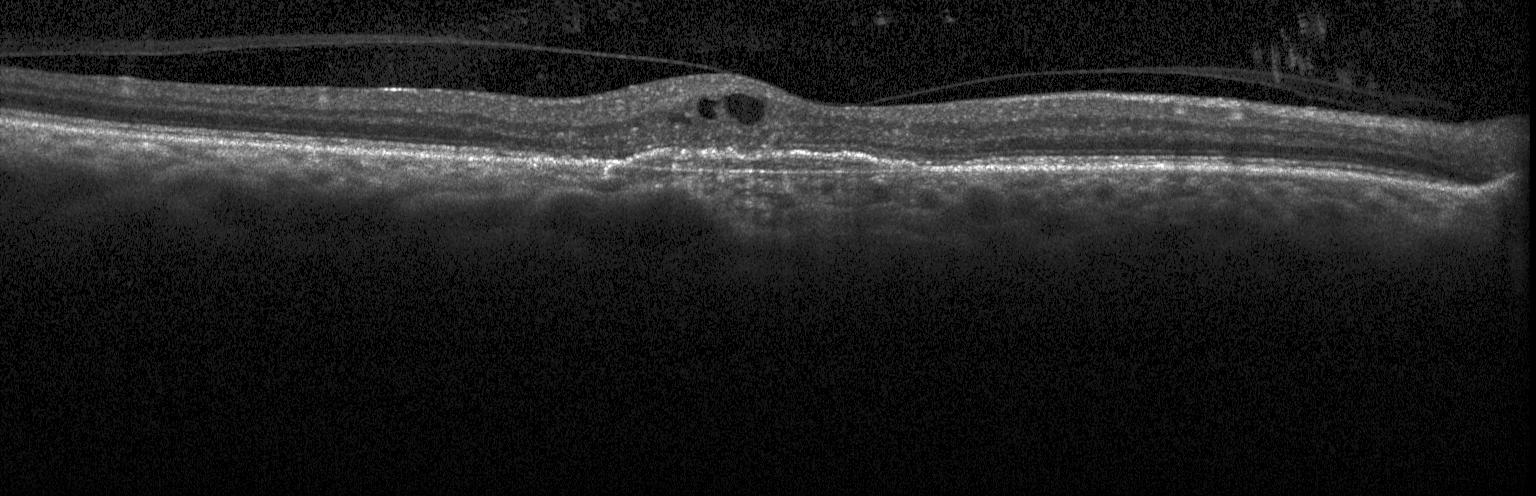

OCT B-scan
Macular OCT: choroidal neovascularization.